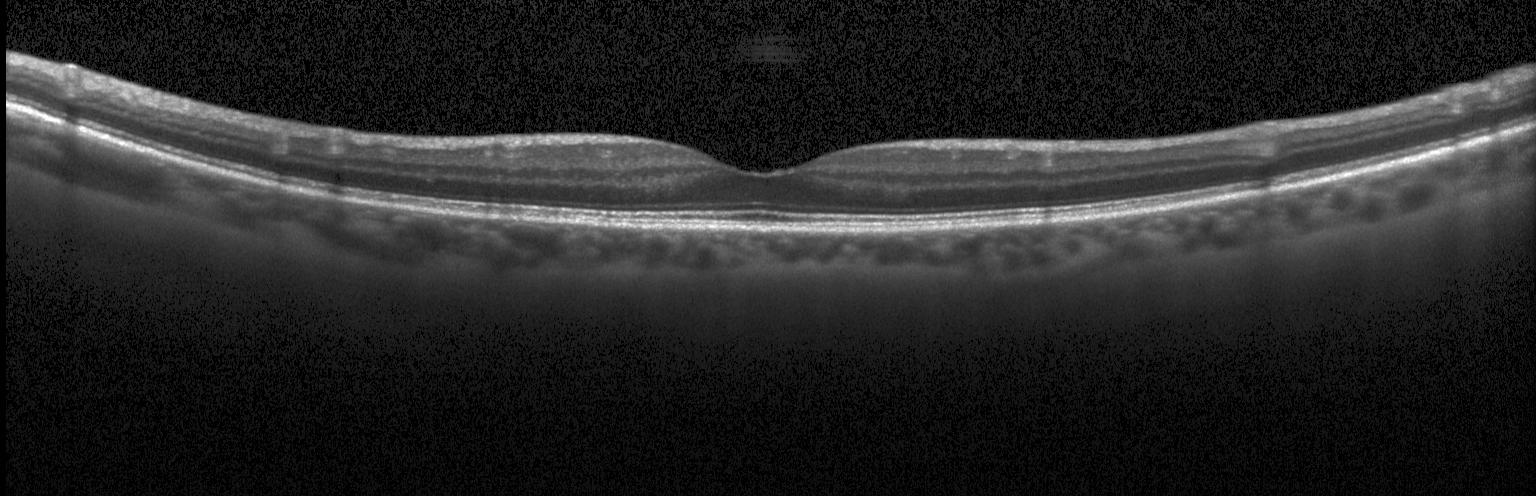 Retinal OCT B-scan · Heidelberg Spectralis. Impression: neither choroidal neovascularization, diabetic macular edema, nor drusen.